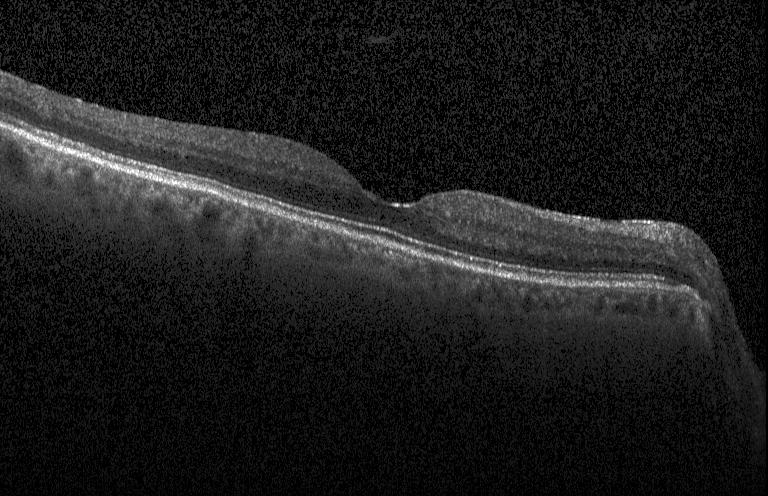 Impression: no evidence of choroidal neovascularization, diabetic macular edema, or drusen.